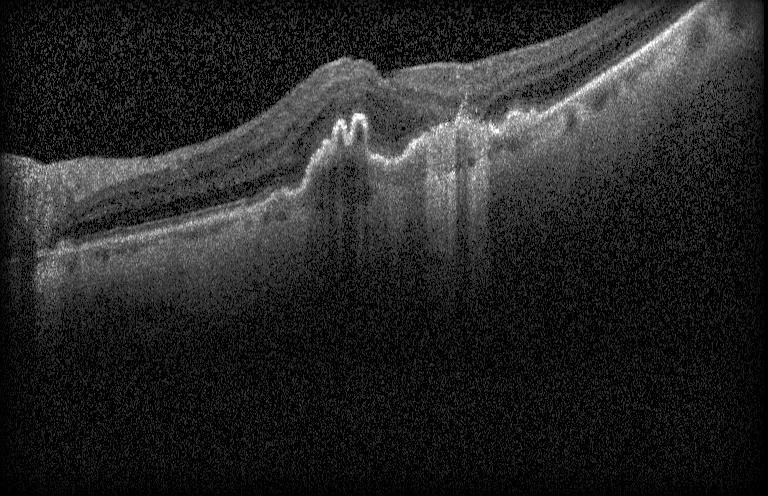
Retinal OCT B-scan.
Choroidal neovascularization (CNV).